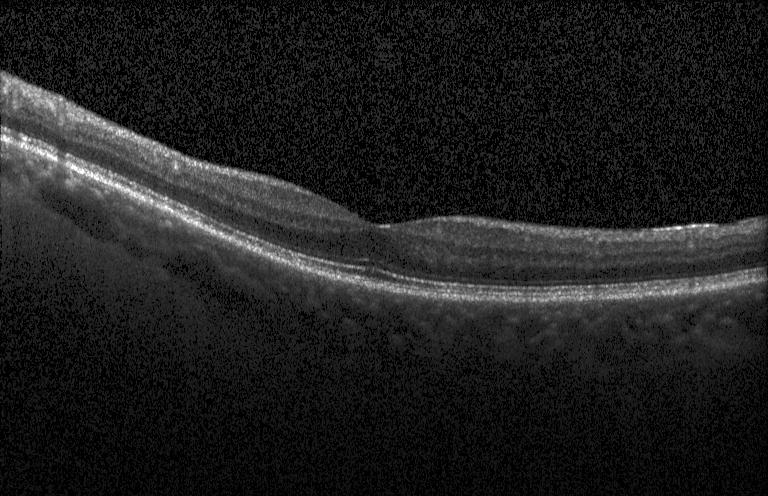

Retinal OCT B-scan. No evidence of choroidal neovascularization, diabetic macular edema, or drusen.